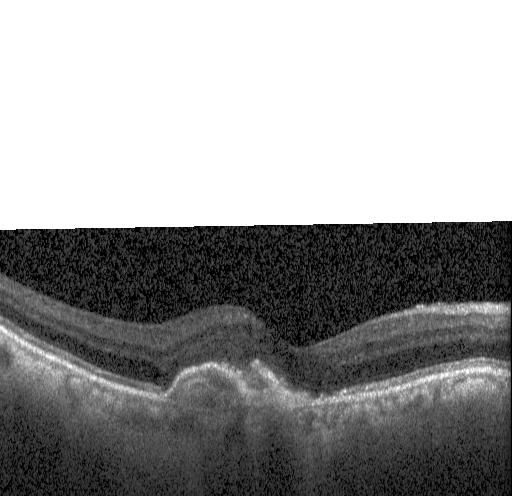
Impression: choroidal neovascularization.